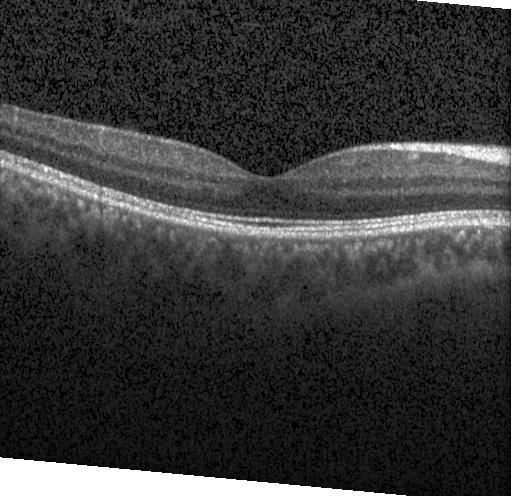

Retinal OCT cross-section; spectral-domain optical coherence tomography.
Impression: neither choroidal neovascularization, diabetic macular edema, nor drusen.